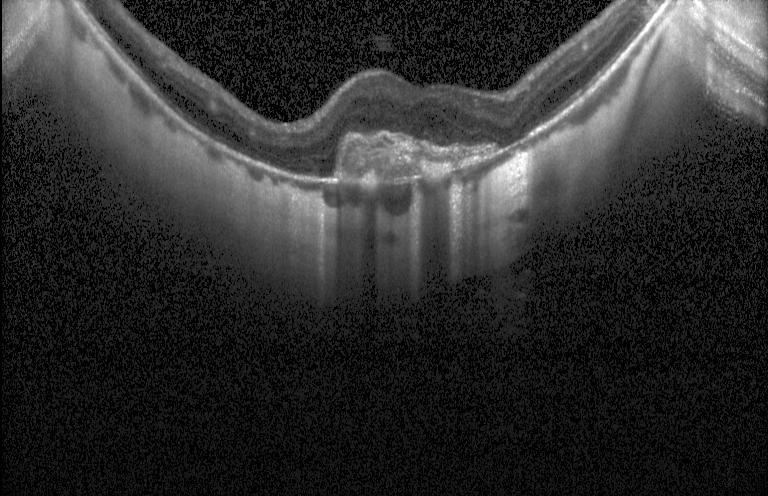 OCT B-scan. A choroidal neovascular membrane.